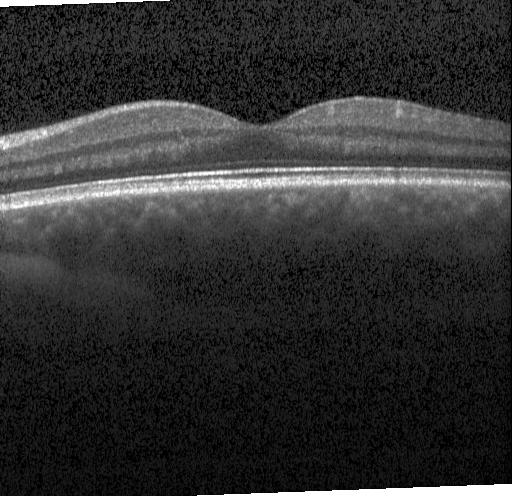
Heidelberg Spectralis; horizontal scan through the fovea; spectral-domain optical coherence tomography; OCT B-scan — This B-scan demonstrates neither choroidal neovascularization, diabetic macular edema, nor drusen.